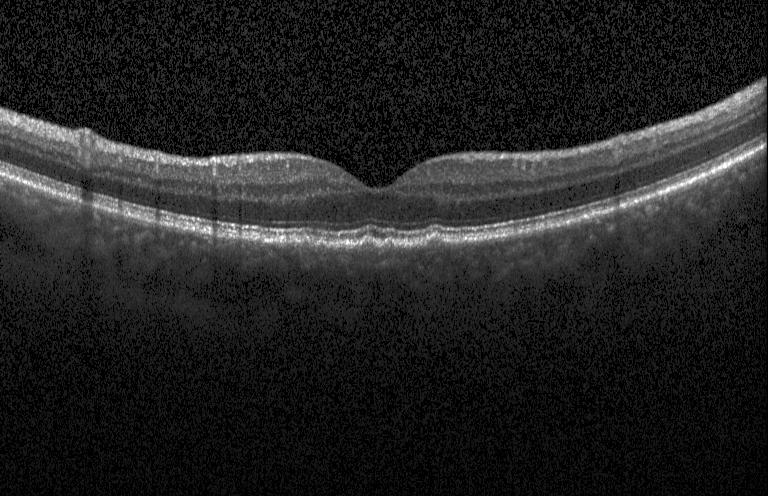 Dx: drusen.